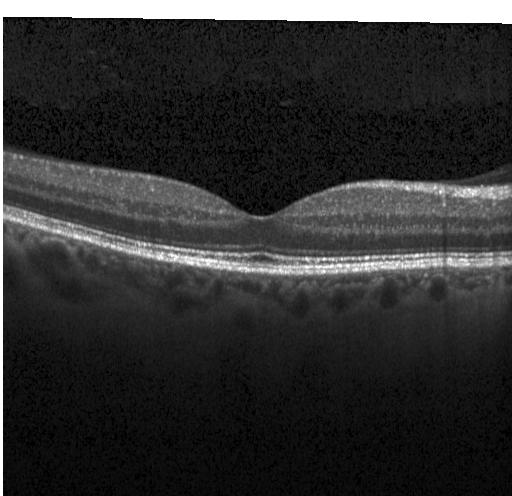

Macular OCT demonstrating no evidence of choroidal neovascularization, diabetic macular edema, or drusen.